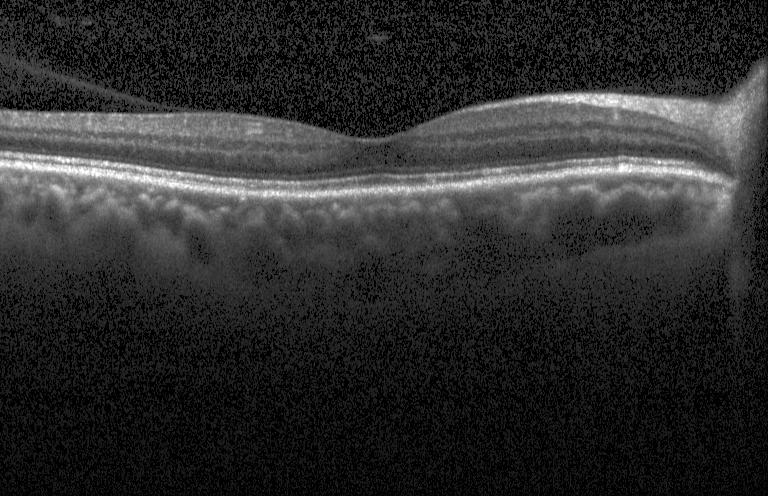

Spectral-domain optical coherence tomography, OCT line scan.
Dx: no choroidal neovascularization, diabetic macular edema, or drusen.